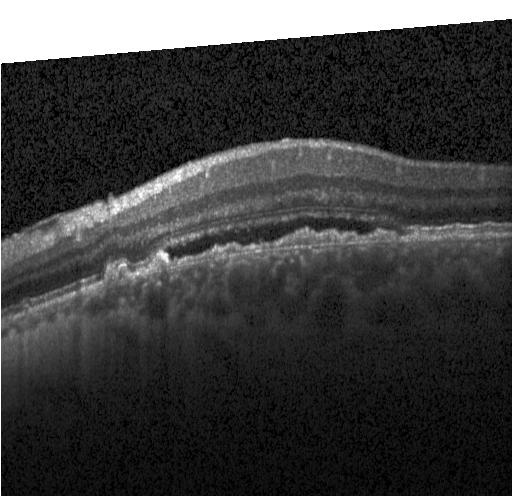

Heidelberg Spectralis OCT system; retinal OCT B-scan.
Impression: a choroidal neovascular membrane.